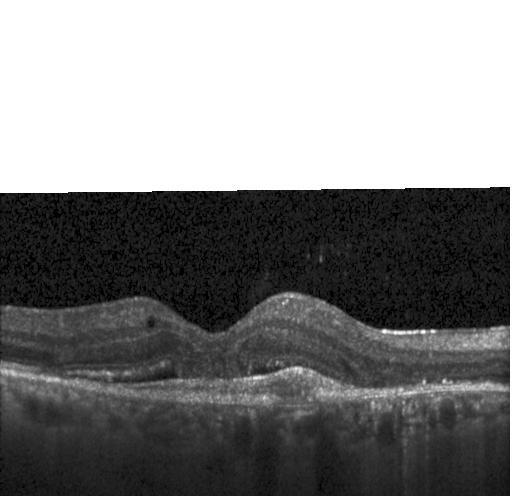
OCT B-scan; macular scan; Heidelberg Spectralis; spectral-domain optical coherence tomography. OCT finding: a choroidal neovascular membrane.